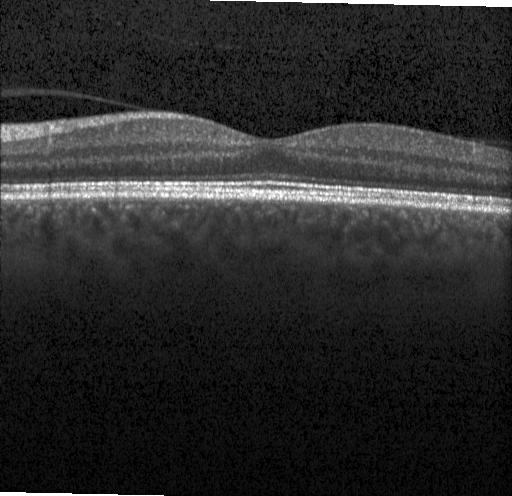
SD-OCT; OCT B-scan; through the macula
Diagnosis: no choroidal neovascularization, diabetic macular edema, or drusen.